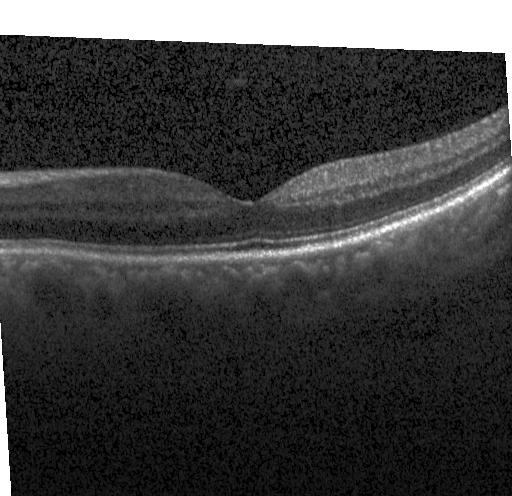
Spectral-domain OCT · retinal OCT cross-section.
Assessment: no choroidal neovascularization, no diabetic macular edema, and no drusen.